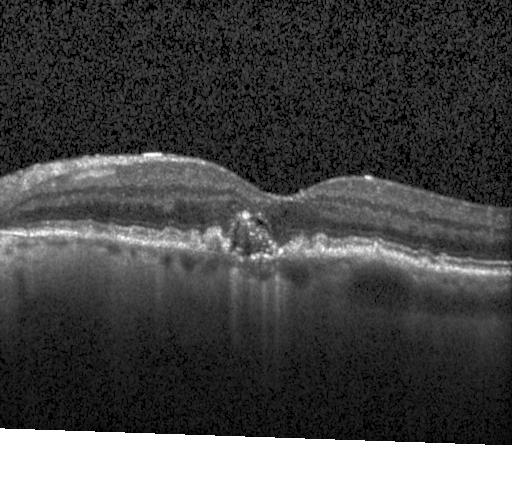
SD-OCT · Heidelberg Spectralis OCT system · optical coherence tomography B-scan · fovea-centered — OCT finding: a choroidal neovascular membrane.